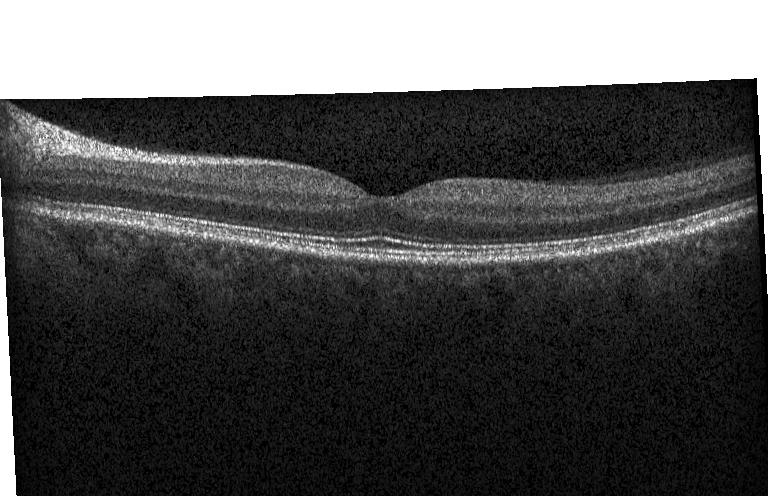

Retinal OCT B-scan.
Dx: no CNV, no DME, and no drusen.